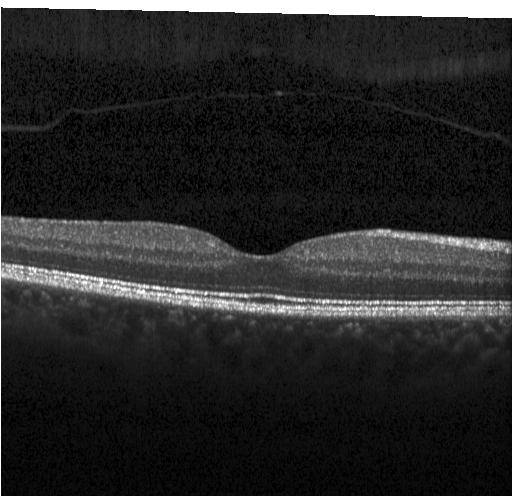 SD-OCT; optical coherence tomography B-scan
Diagnosis: no evidence of choroidal neovascularization, diabetic macular edema, or drusen.